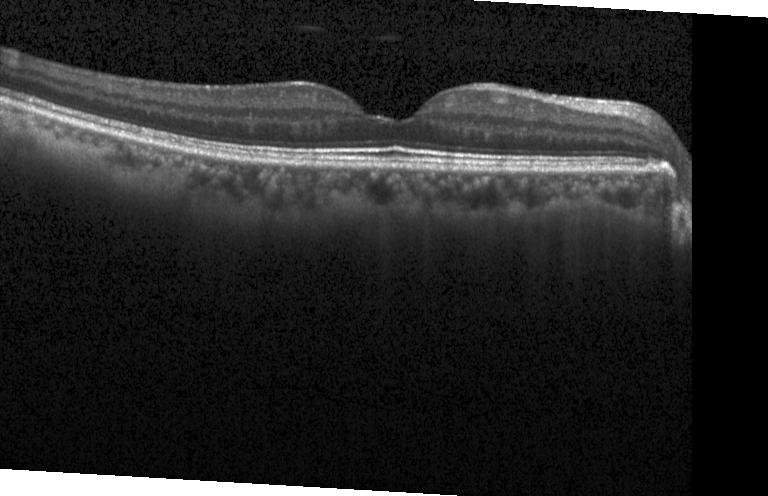
OCT B-scan. Spectral-domain OCT. Finding: no evidence of choroidal neovascularization, diabetic macular edema, or drusen.